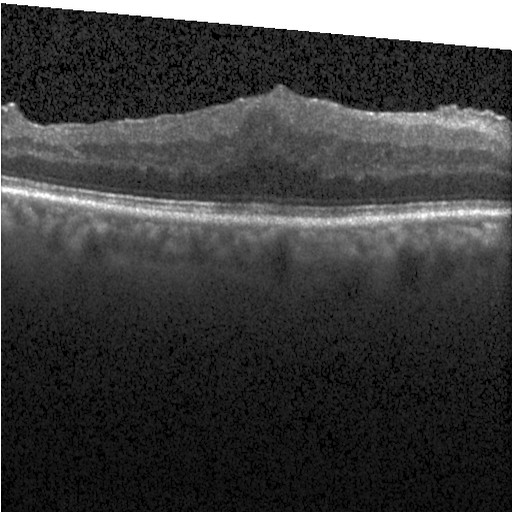 Macular OCT demonstrating diabetic macular edema.